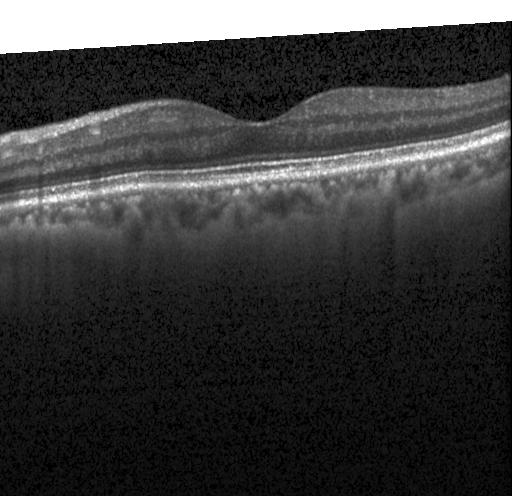
Spectral-domain OCT B-scan: neither CNV, DME, nor drusen.